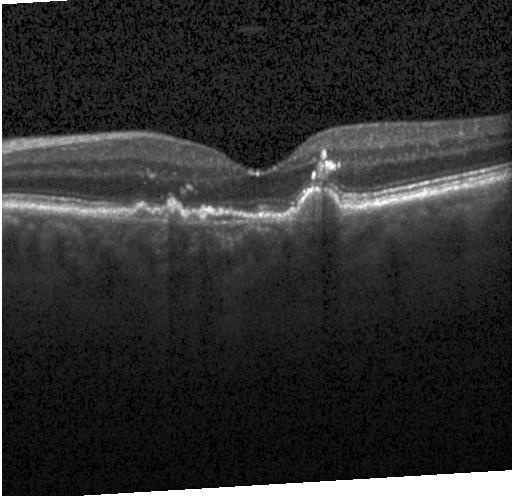 Diagnosis: a choroidal neovascular membrane.